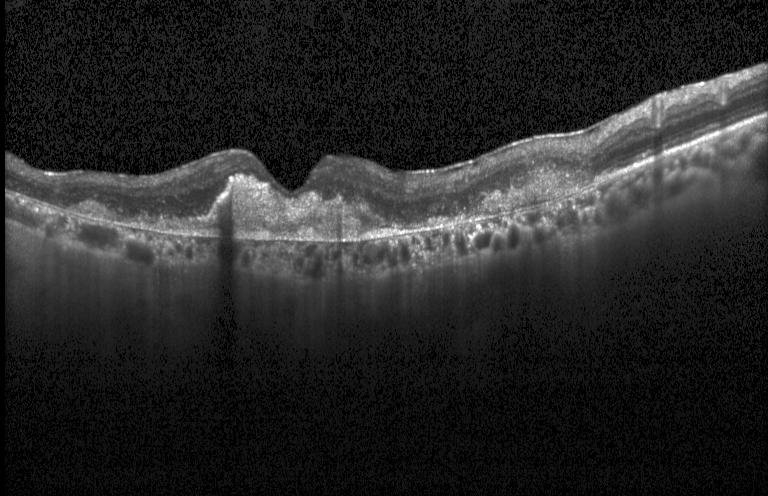
OCT finding: choroidal neovascularization.